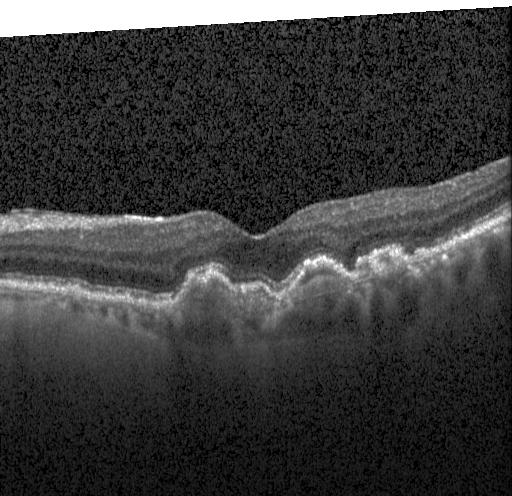 Through the macula. Optical coherence tomography scan. Spectral-domain OCT — Finding: a choroidal neovascular membrane.